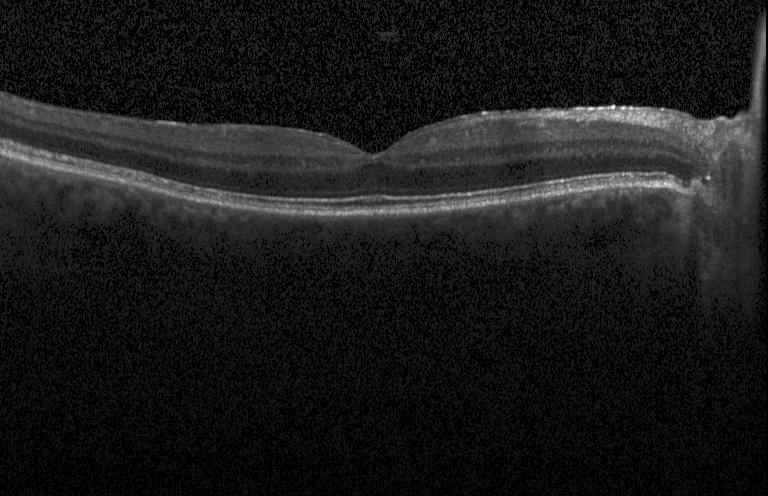

Impression: neither choroidal neovascularization, diabetic macular edema, nor drusen.